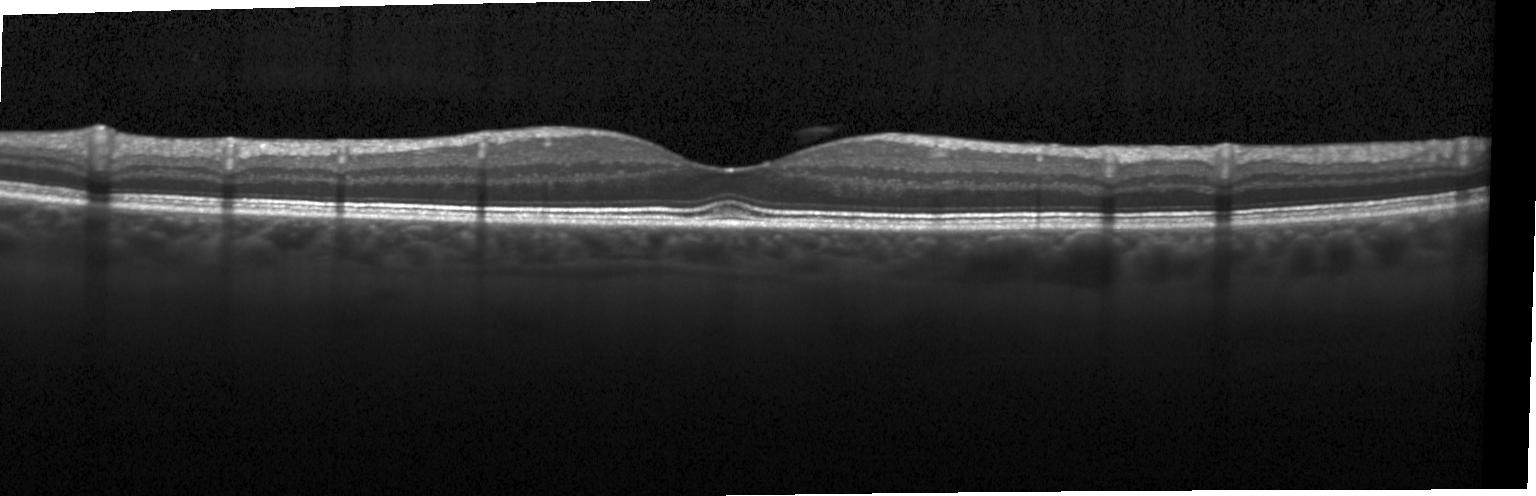

Optical coherence tomography B-scan.
Macular OCT: no evidence of choroidal neovascularization, diabetic macular edema, or drusen.